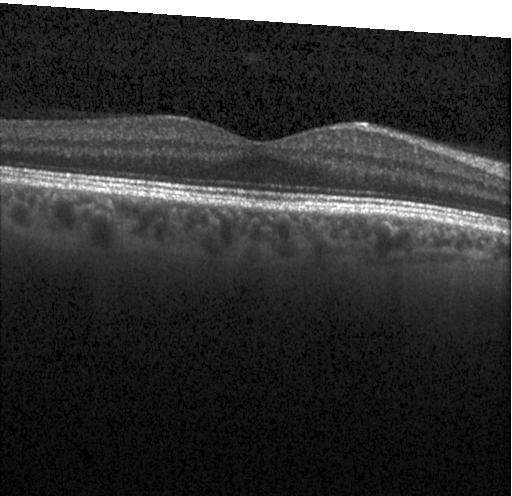 Fovea-centered; optical coherence tomography B-scan — Finding: no choroidal neovascularization, no diabetic macular edema, and no drusen.